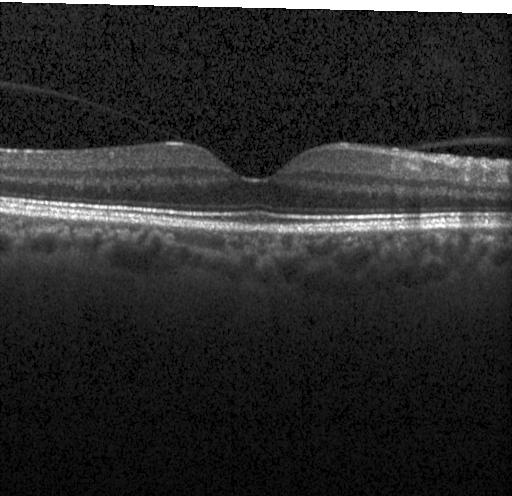 Finding: neither choroidal neovascularization, diabetic macular edema, nor drusen.